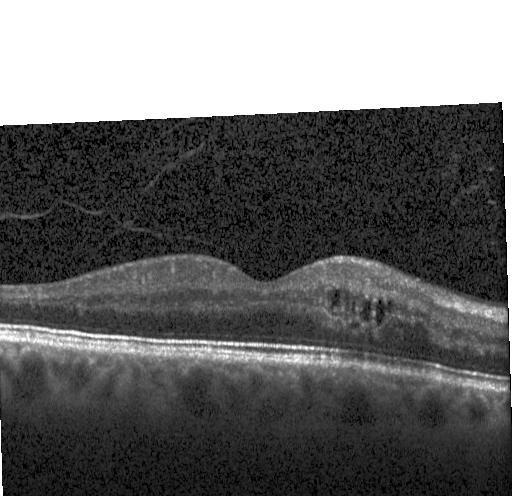 Retinal OCT cross-section · instrument: Heidelberg Spectralis · fovea-centered.
DME.